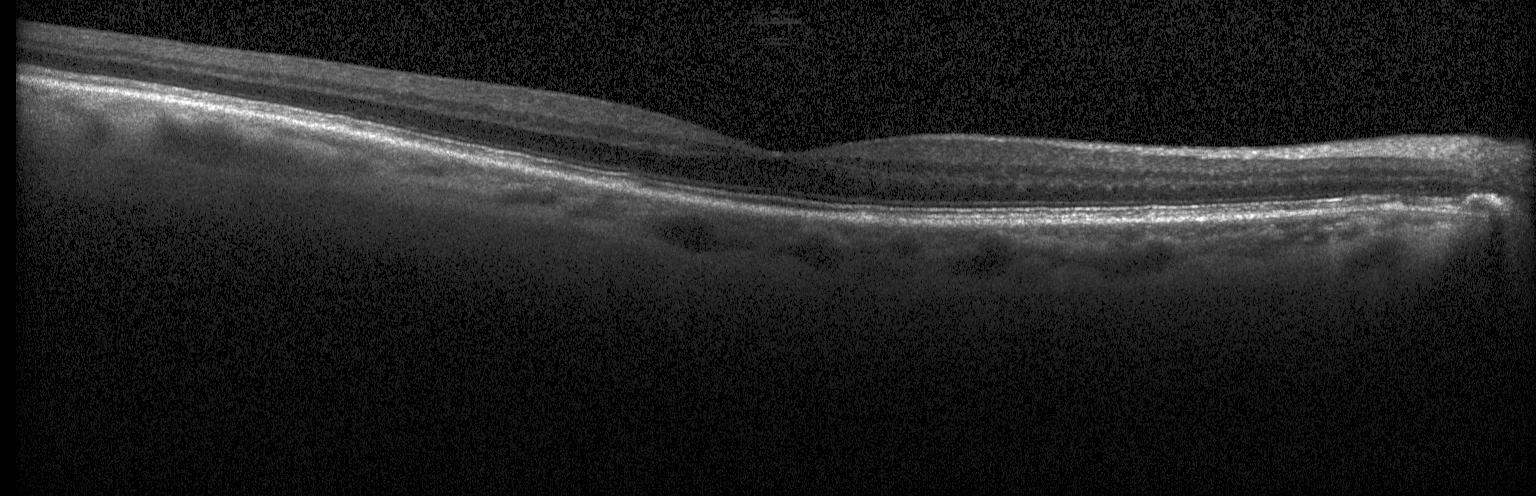 The scan shows no choroidal neovascularization, no diabetic macular edema, and no drusen.